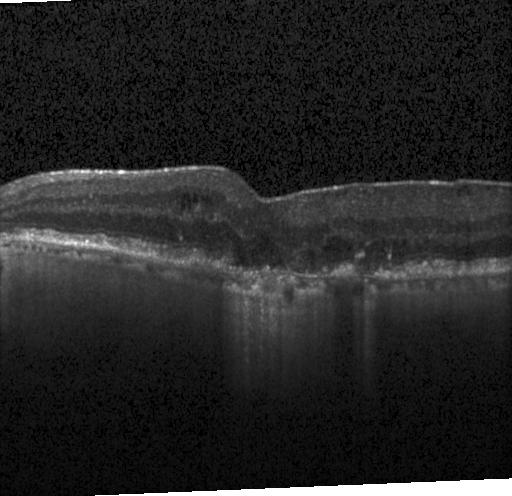

Retinal OCT B-scan. Macular scan
Impression: choroidal neovascularization.